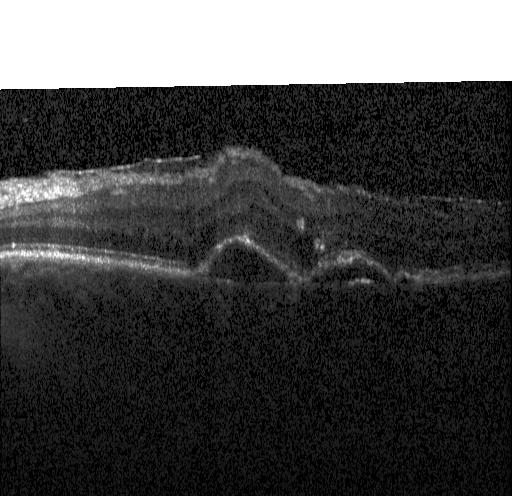

Optical coherence tomography scan — Diagnosis: choroidal neovascularization.